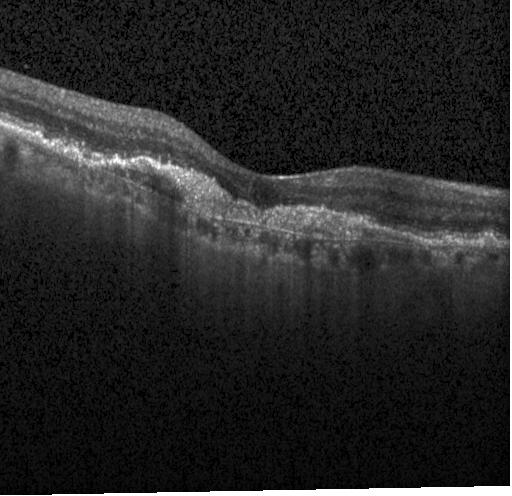
Acquired on a Heidelberg Spectralis, macular scan, spectral-domain OCT, retinal OCT cross-section — Impression: a choroidal neovascular membrane.